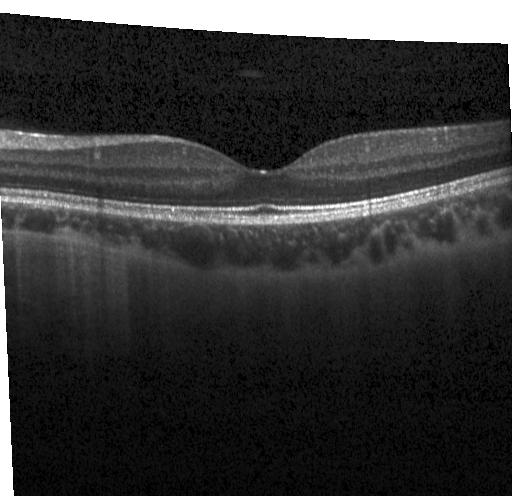

SD-OCT; acquired on a Heidelberg Spectralis; OCT B-scan. Assessment: no choroidal neovascularization, no diabetic macular edema, and no drusen.